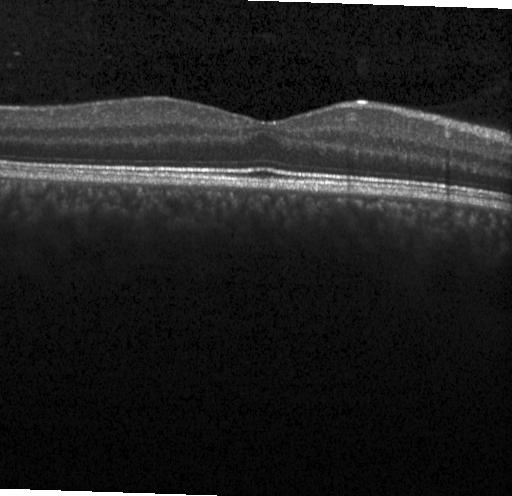

This B-scan demonstrates no evidence of choroidal neovascularization, diabetic macular edema, or drusen.